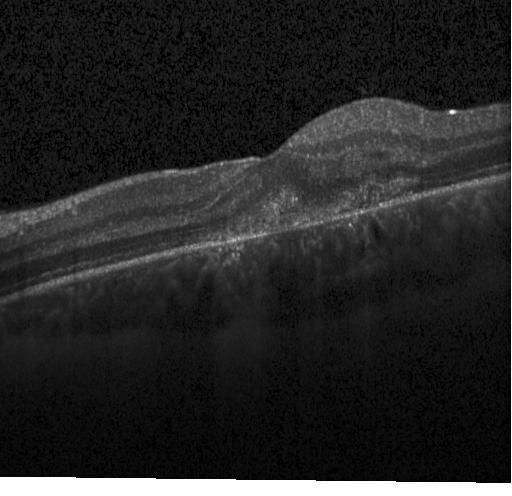 Diagnosis: a choroidal neovascular membrane.